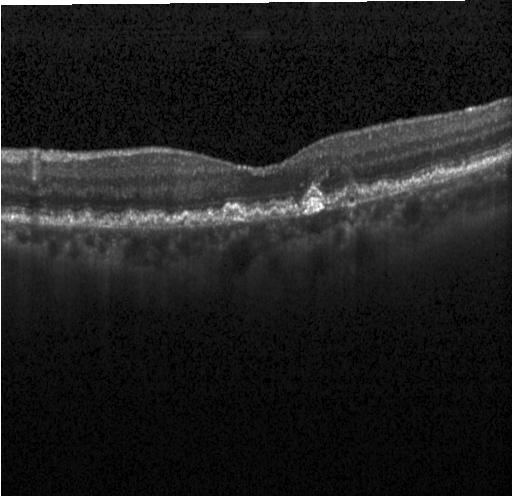
Optical coherence tomography B-scan, spectral-domain OCT
Finding: sub-RPE drusenoid deposits.